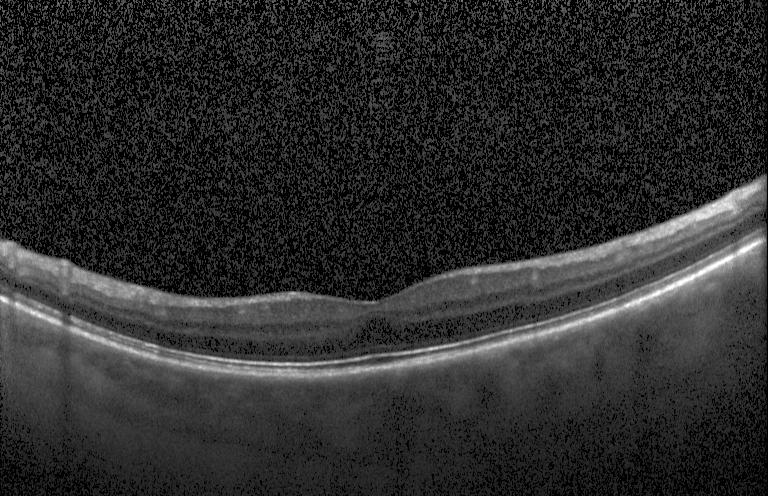 Horizontal scan through the fovea · acquired on a Heidelberg Spectralis · retinal OCT cross-section
Impression: no evidence of choroidal neovascularization, diabetic macular edema, or drusen.